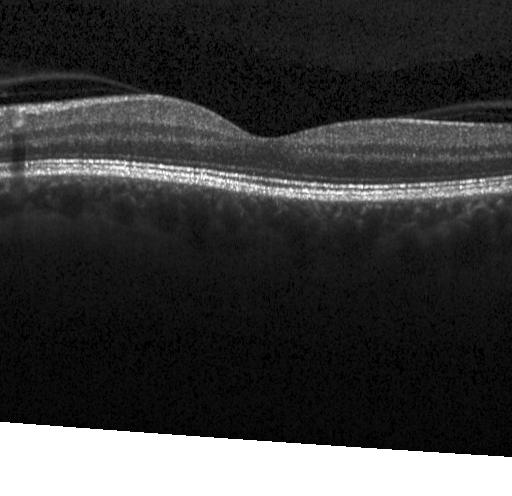 Optical coherence tomography B-scan. Heidelberg Spectralis OCT system — Diagnosis: no choroidal neovascularization, diabetic macular edema, or drusen.